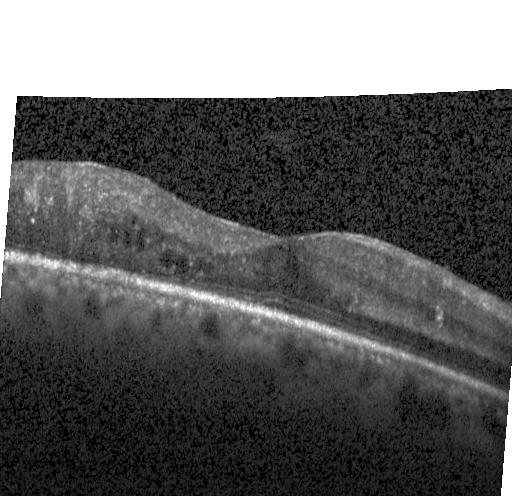

Instrument: Heidelberg Spectralis, OCT B-scan, centered on the fovea, spectral-domain OCT.
Diabetic macular edema (DME).